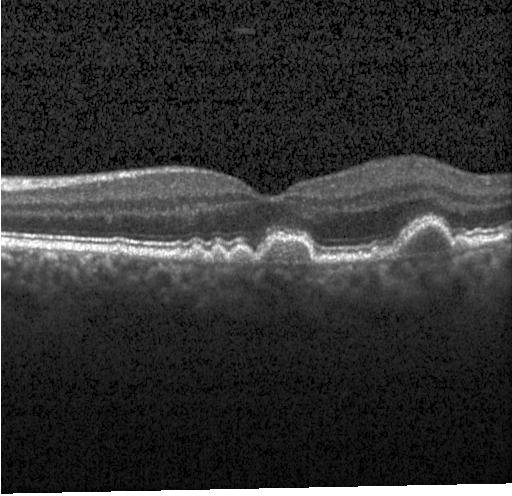 Spectral-domain OCT B-scan: multiple drusen.